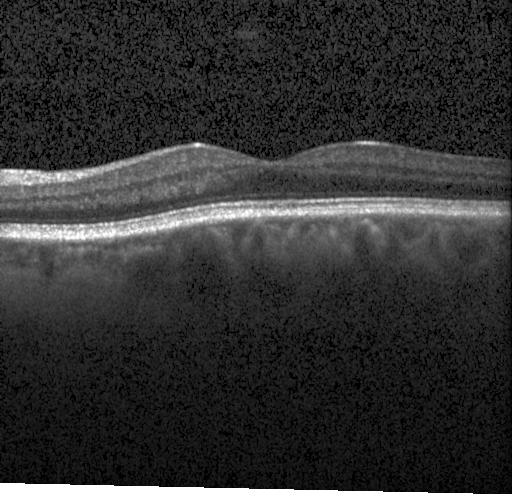
Macular scan, SD-OCT, retinal OCT B-scan. Diagnosis: no evidence of choroidal neovascularization, diabetic macular edema, or drusen.